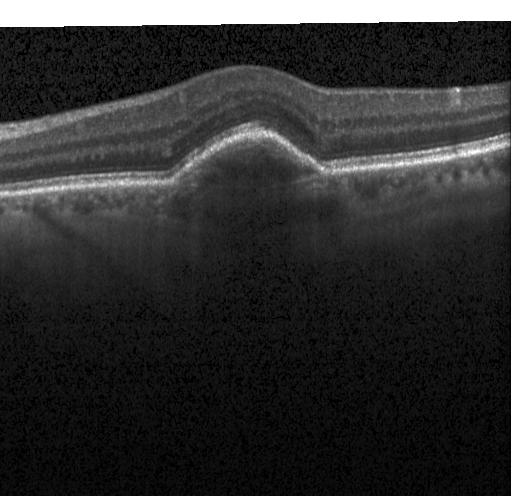 Through the macula, Heidelberg Spectralis, retinal OCT B-scan
Diagnosis: a choroidal neovascular membrane.